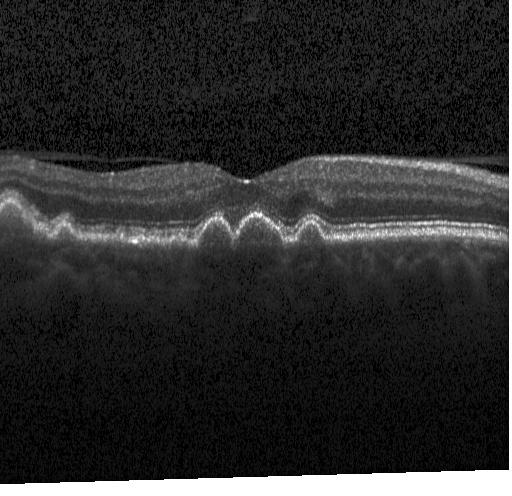 Retinal OCT cross-section showing drusen.